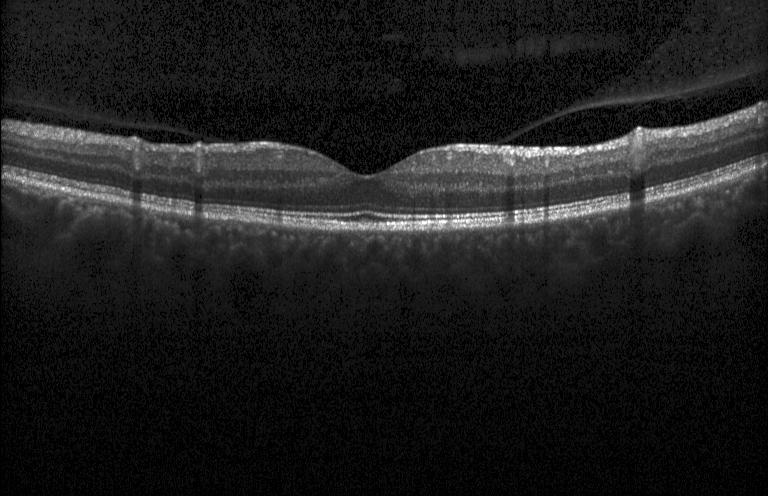

Macular OCT: no evidence of CNV, DME, or drusen.